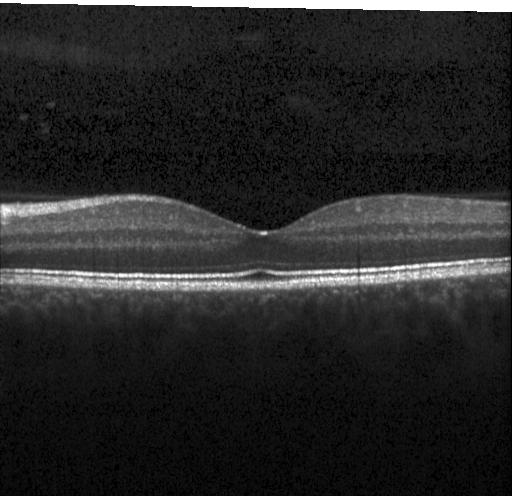
Through the macula. Spectral-domain OCT. Retinal OCT B-scan. Heidelberg Spectralis OCT system.
The scan shows no evidence of CNV, DME, or drusen.